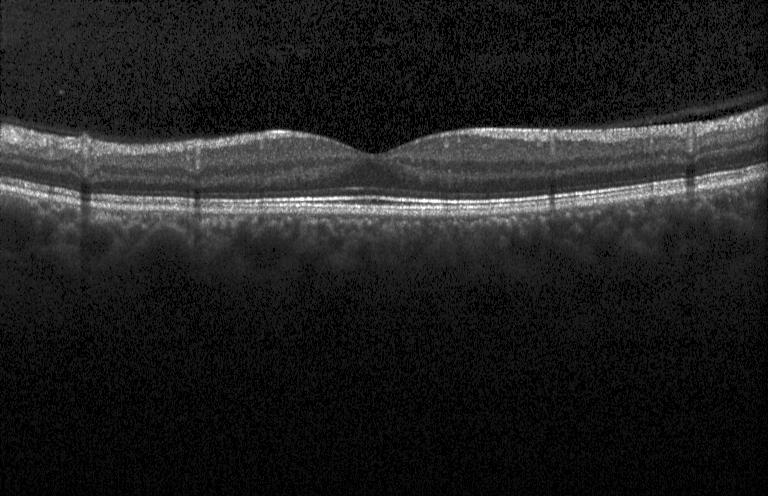 Macular OCT demonstrating no evidence of CNV, DME, or drusen.